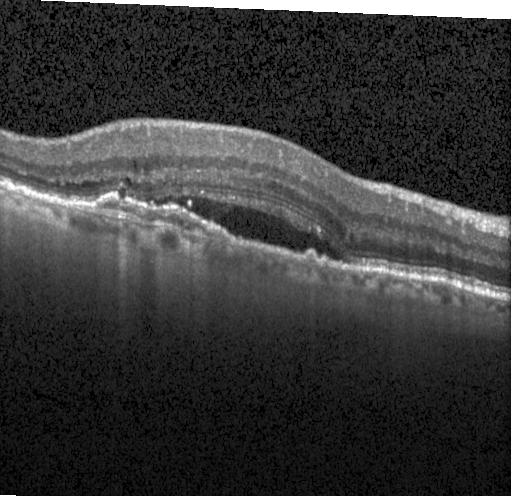

Macular OCT: choroidal neovascularization (CNV).